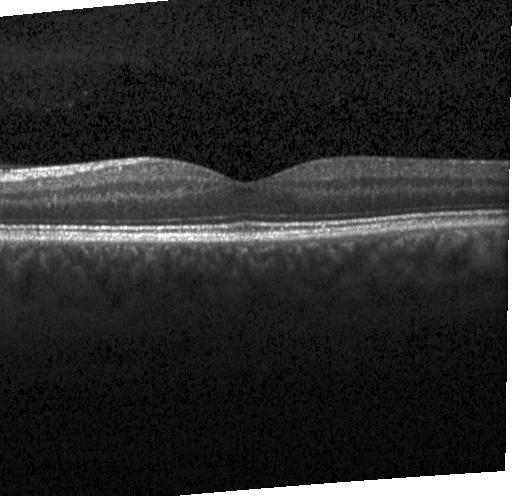 Retinal OCT cross-section. SD-OCT. Instrument: Heidelberg Spectralis. Impression: no evidence of choroidal neovascularization, diabetic macular edema, or drusen.